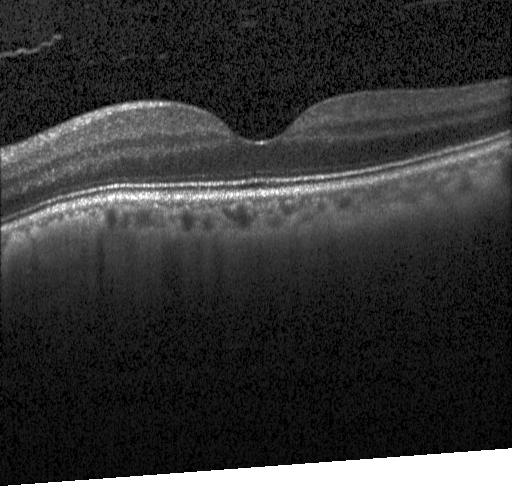
Diagnosis: no CNV, no DME, and no drusen.